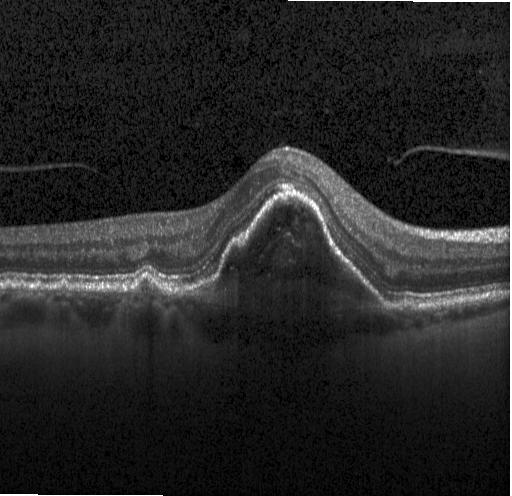

Optical coherence tomography scan. Impression: a choroidal neovascular membrane.